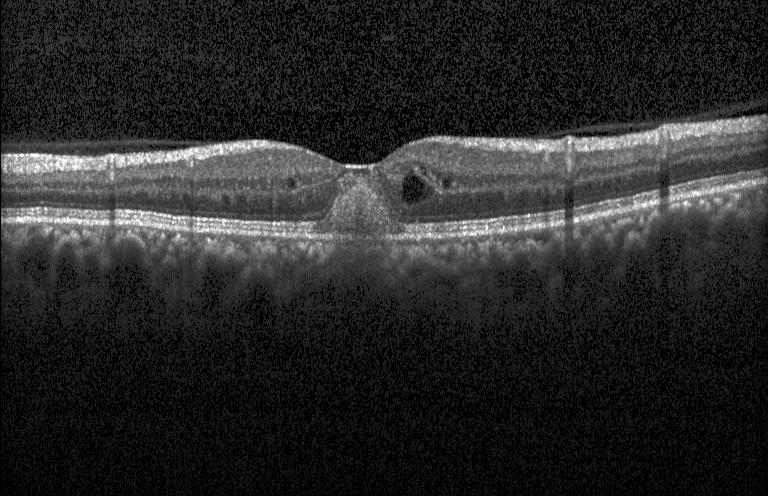

Spectral-domain optical coherence tomography, OCT line scan, macular scan, instrument: Heidelberg Spectralis. Impression: a choroidal neovascular membrane.